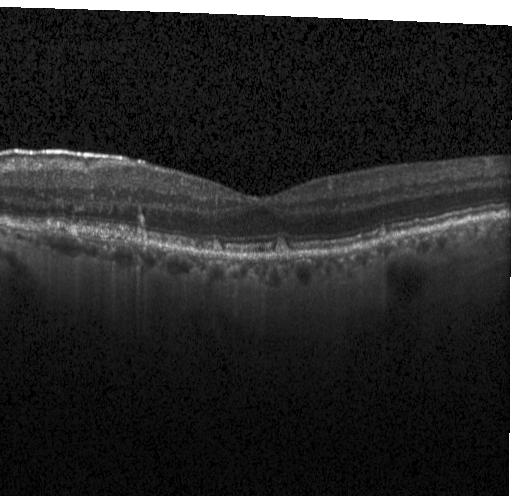 The scan shows drusen.